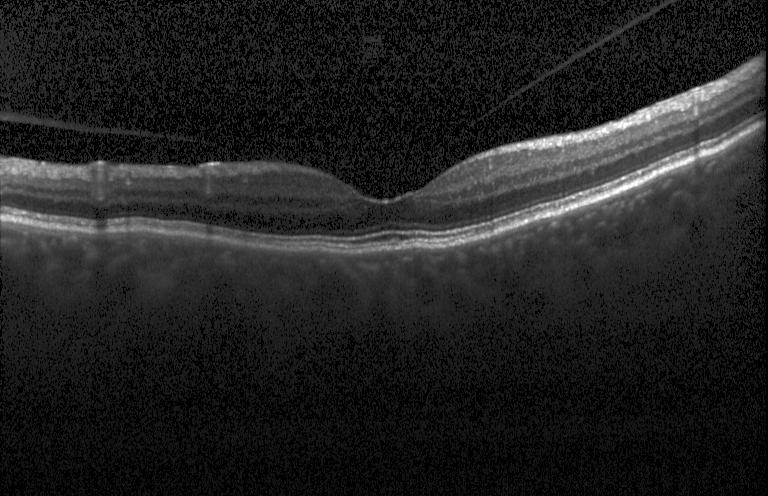
Horizontal scan through the fovea · OCT line scan · SD-OCT
Assessment: no evidence of choroidal neovascularization, diabetic macular edema, or drusen.